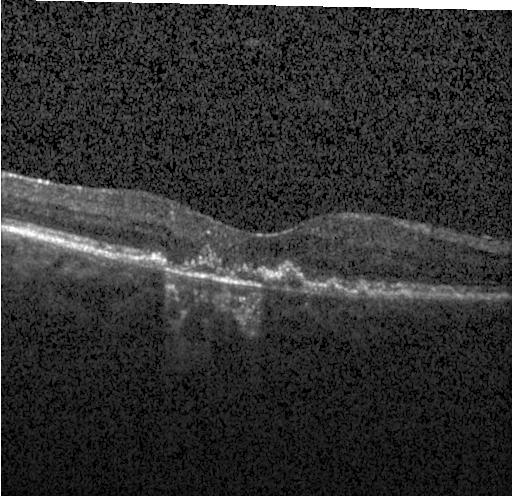 OCT finding: choroidal neovascularization.